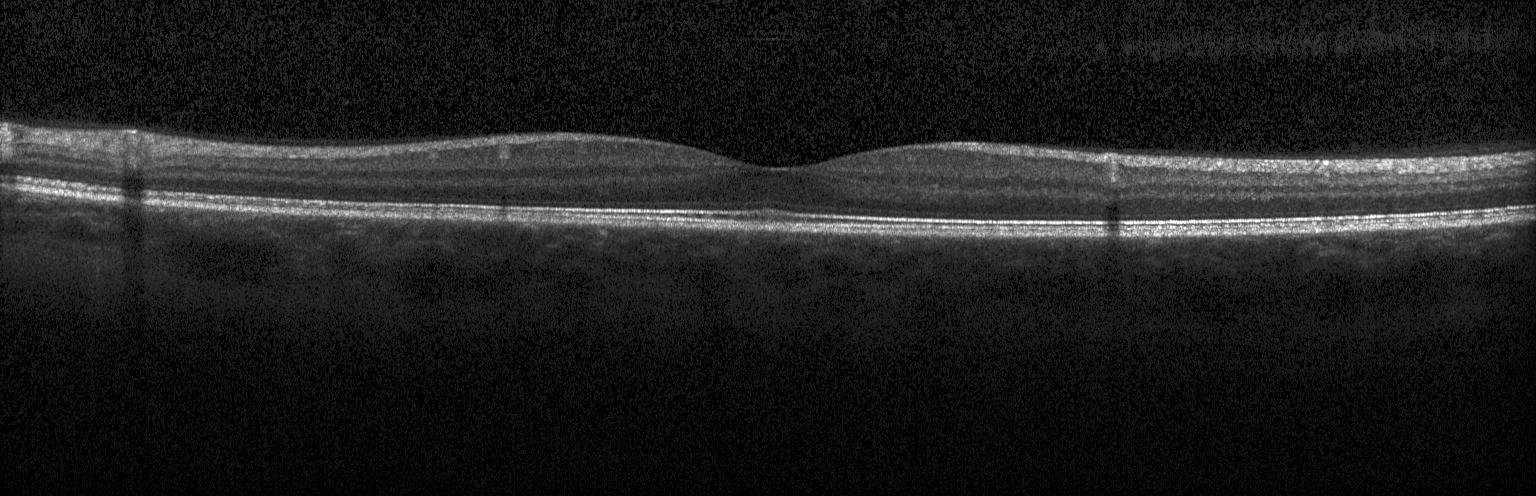 Heidelberg Spectralis OCT system; OCT B-scan
Impression: no evidence of choroidal neovascularization, diabetic macular edema, or drusen.